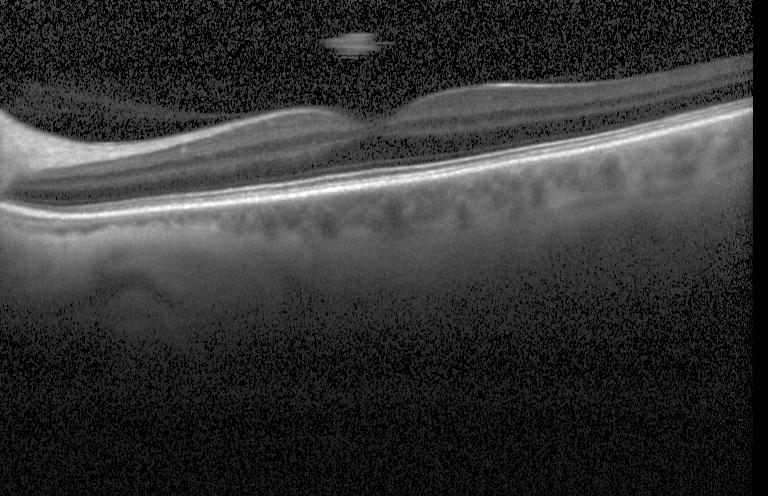
Retinal OCT B-scan — Impression: no CNV, DME, or drusen.